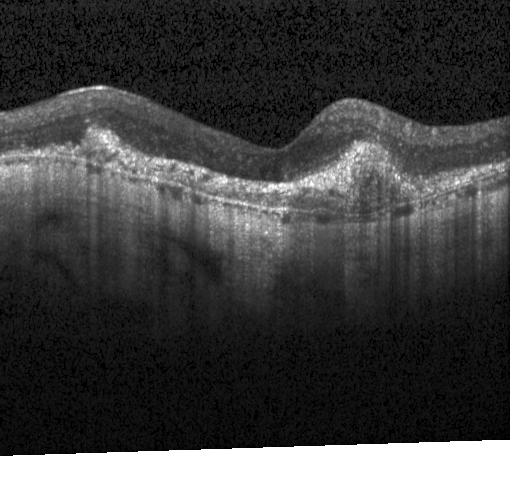
Horizontal scan through the fovea · spectral-domain OCT · instrument: Heidelberg Spectralis · retinal OCT cross-section. Finding: a choroidal neovascular membrane.